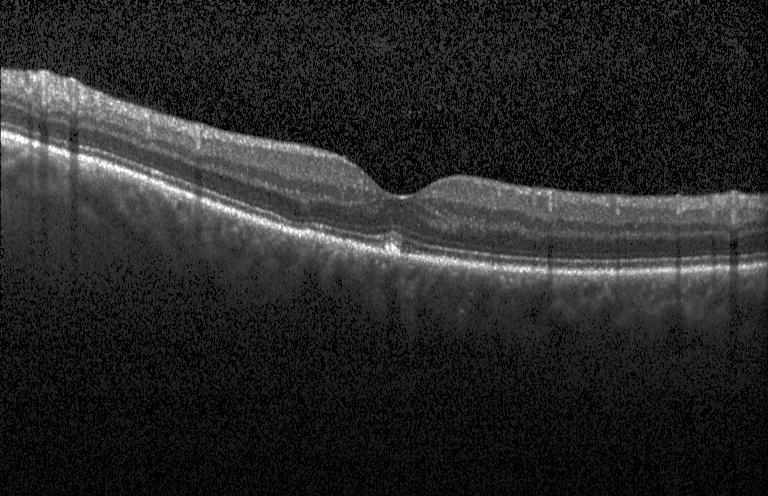 Assessment: drusen.